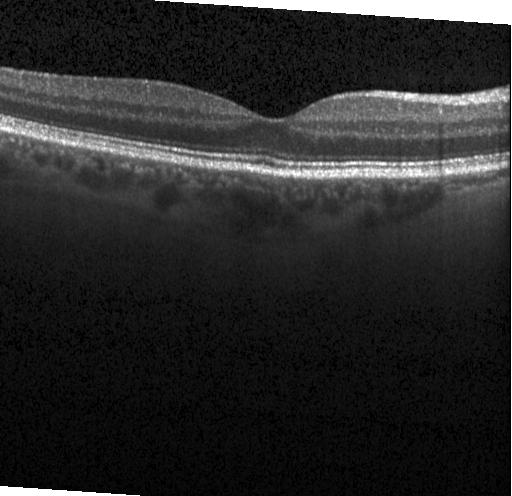

Finding: no choroidal neovascularization, diabetic macular edema, or drusen.